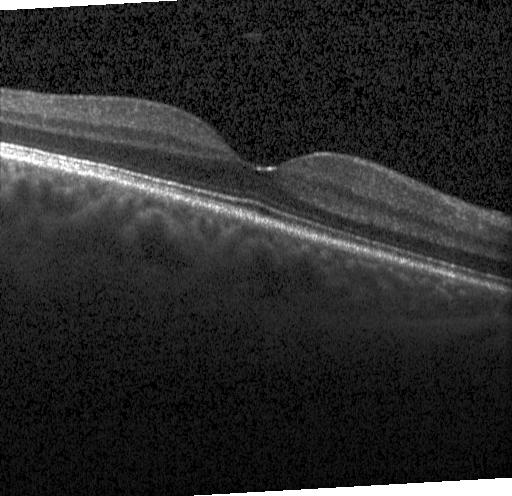 OCT scan showing no choroidal neovascularization, diabetic macular edema, or drusen.